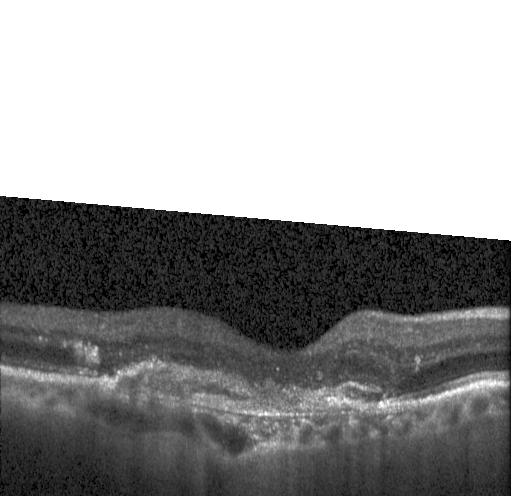

Finding: a choroidal neovascular membrane.